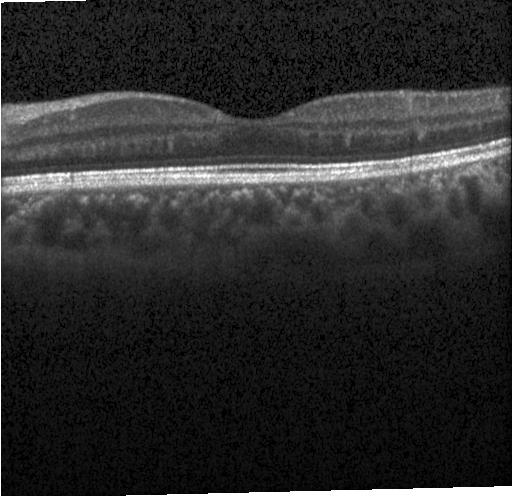
OCT B-scan. Assessment: no evidence of choroidal neovascularization, diabetic macular edema, or drusen.